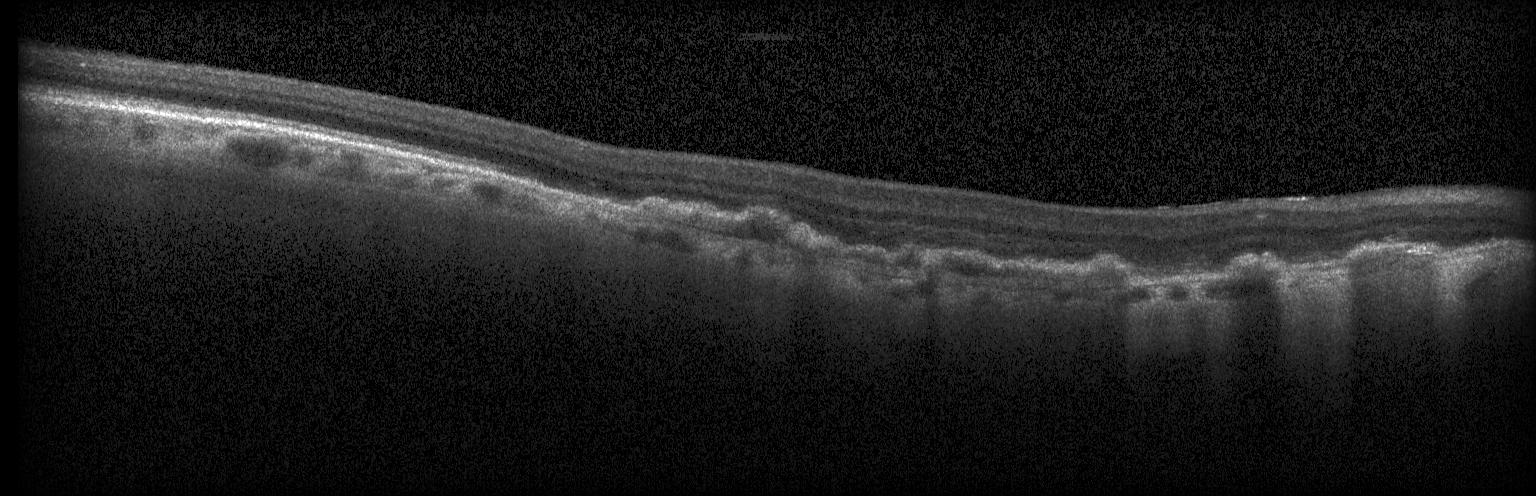 Optical coherence tomography B-scan — Assessment: a choroidal neovascular membrane.